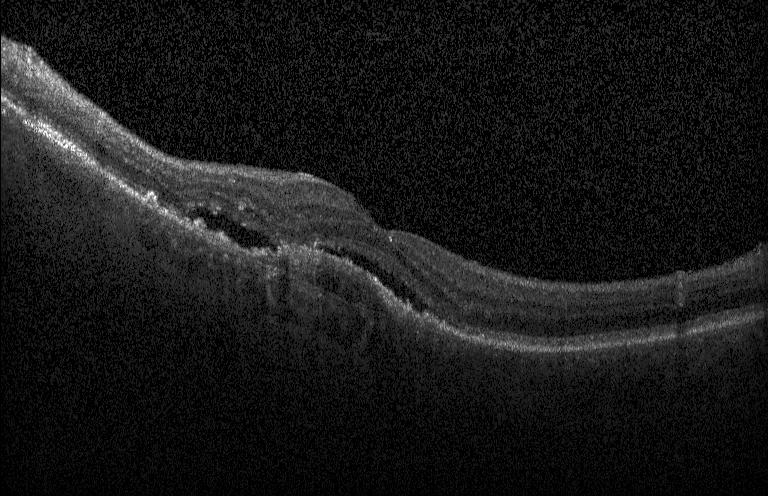

Finding: a choroidal neovascular membrane.